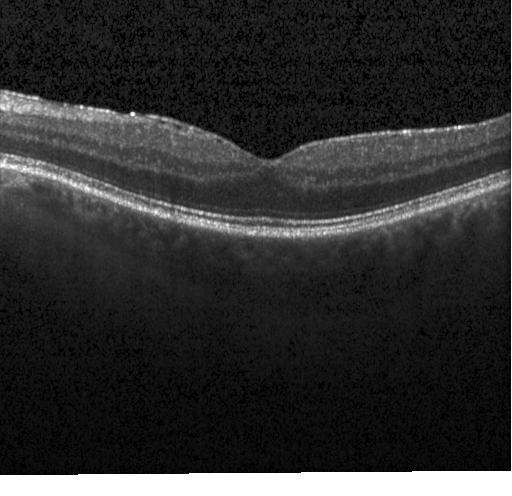

Retinal OCT B-scan — Impression: no choroidal neovascularization, no diabetic macular edema, and no drusen.